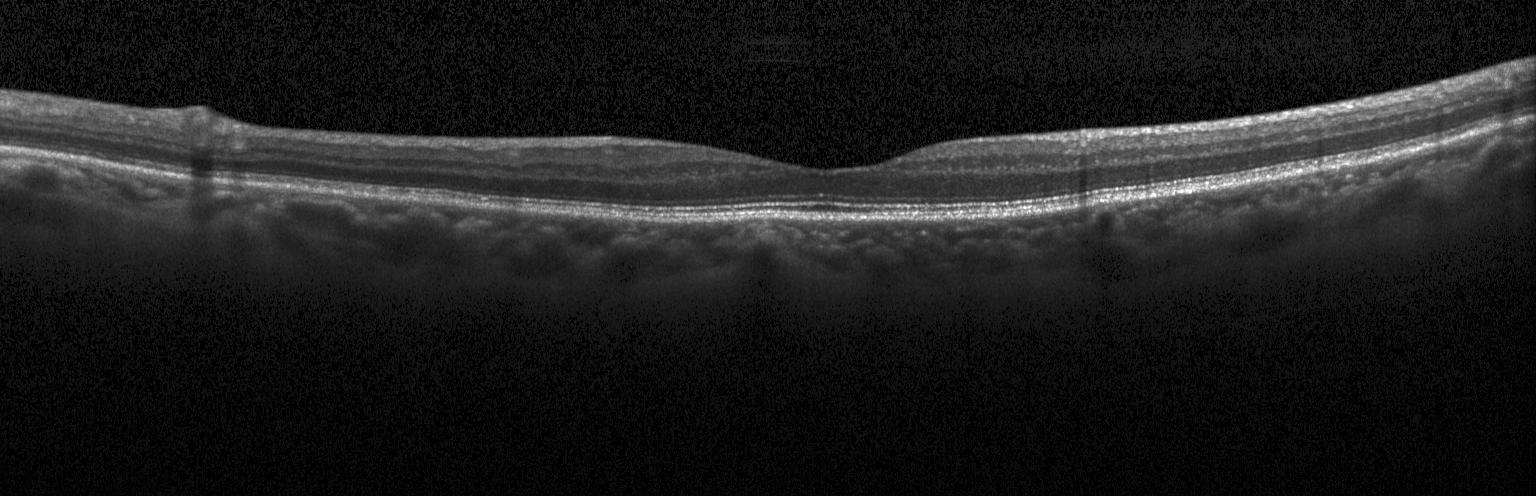
OCT B-scan — Dx: neither CNV, DME, nor drusen.